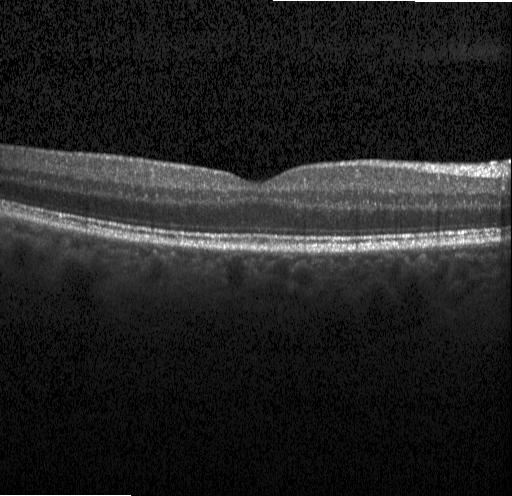 Instrument: Heidelberg Spectralis; retinal OCT cross-section — No choroidal neovascularization, no diabetic macular edema, and no drusen.